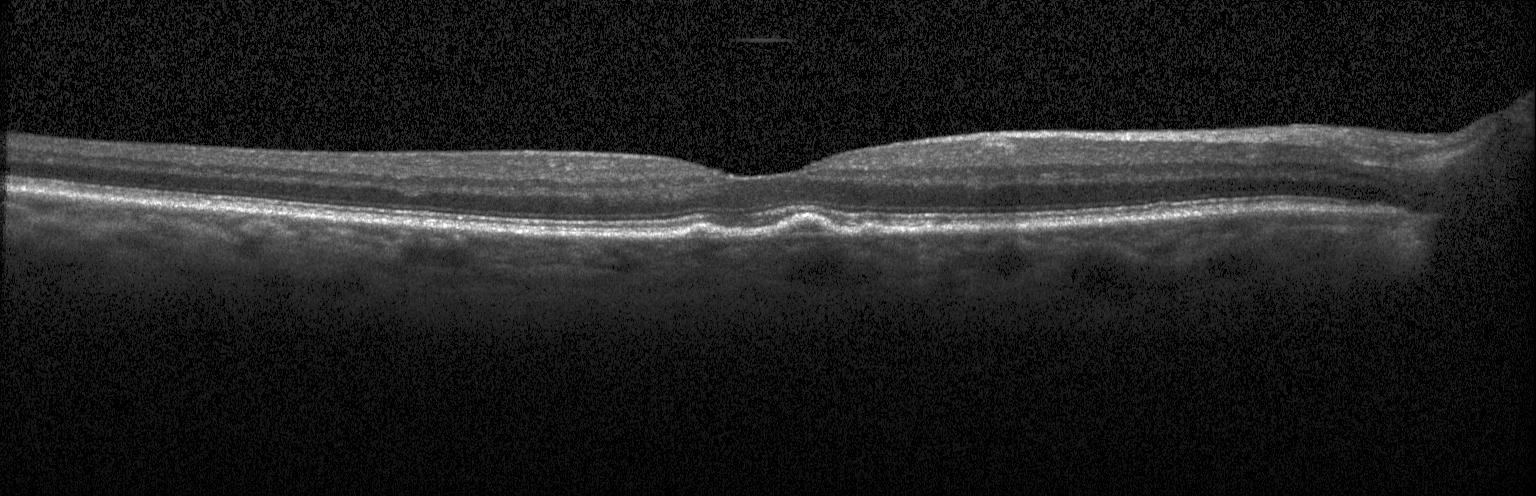

OCT line scan, fovea-centered — Diagnosis: drusen.